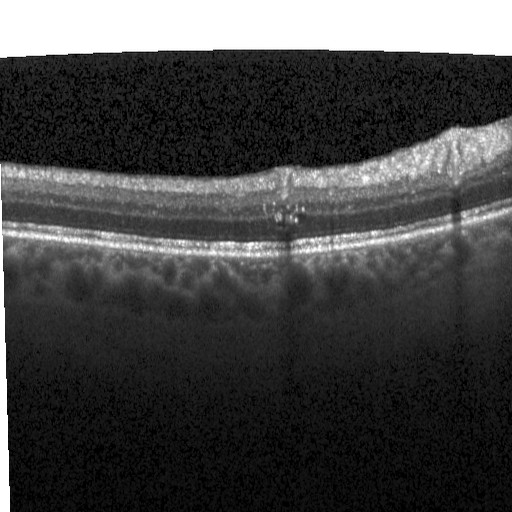 Dx: diabetic macular edema.